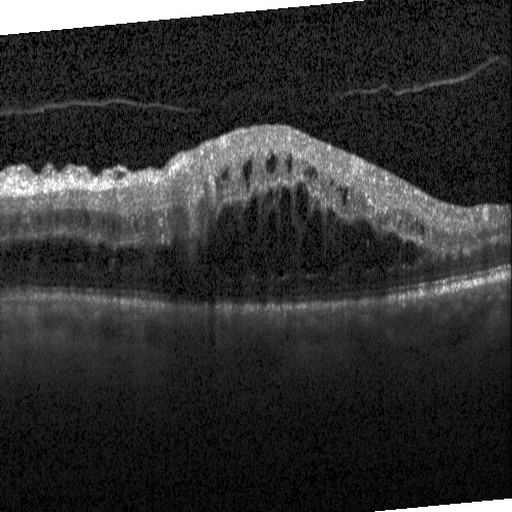
Centered on the fovea · OCT line scan. OCT finding: diabetic macular edema.